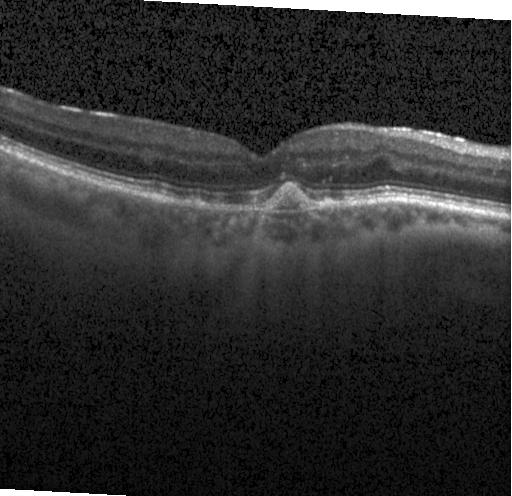 Impression: choroidal neovascularization (CNV).